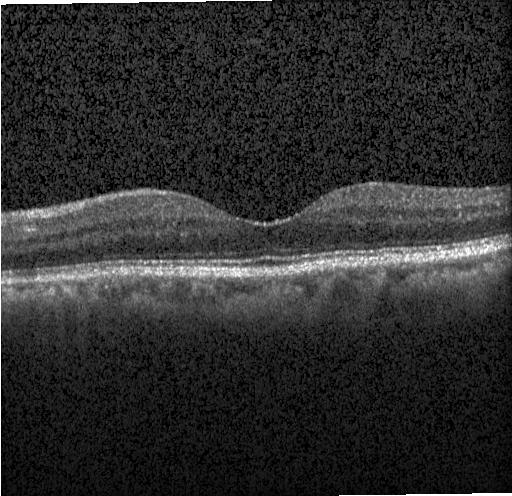 Heidelberg Spectralis. Optical coherence tomography scan. SD-OCT. Through the macula.
Macular OCT: neither choroidal neovascularization, diabetic macular edema, nor drusen.